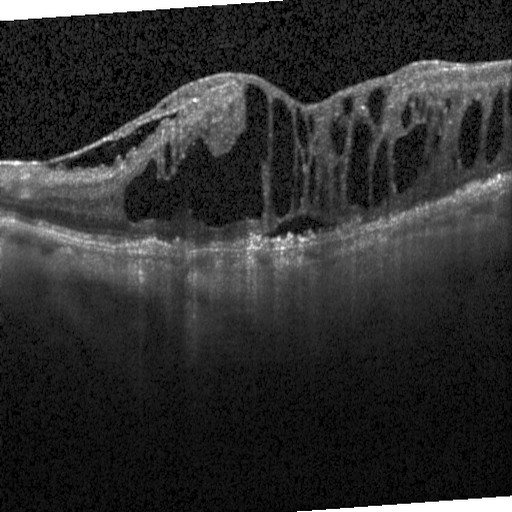

Finding: diabetic macular edema (DME).